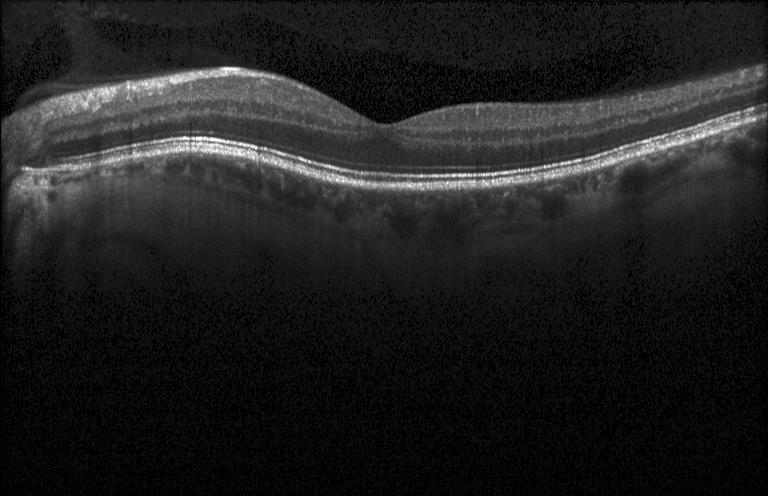

Fovea-centered. OCT line scan — Impression: no choroidal neovascularization, no diabetic macular edema, and no drusen.